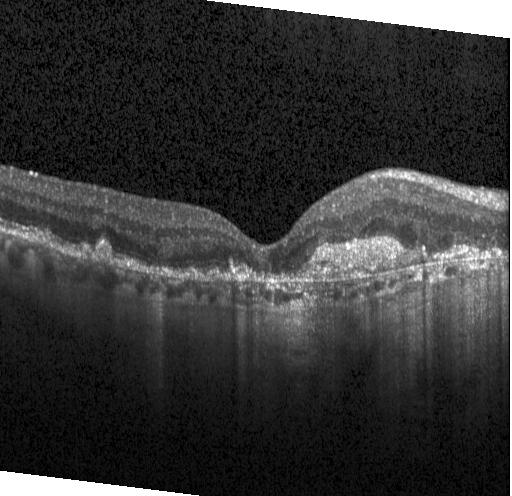
Finding: choroidal neovascularization.